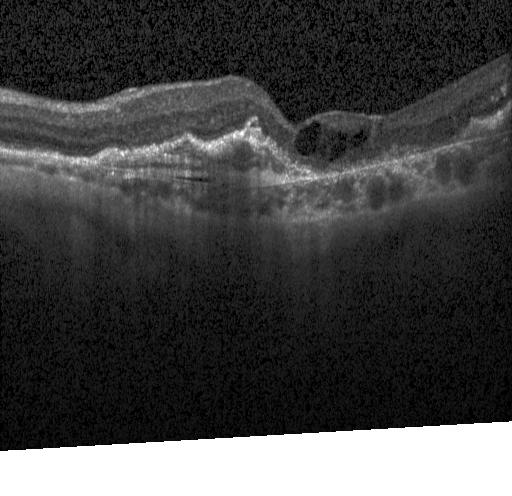
Fovea-centered, instrument: Heidelberg Spectralis, optical coherence tomography scan, spectral-domain optical coherence tomography. Finding: a choroidal neovascular membrane.